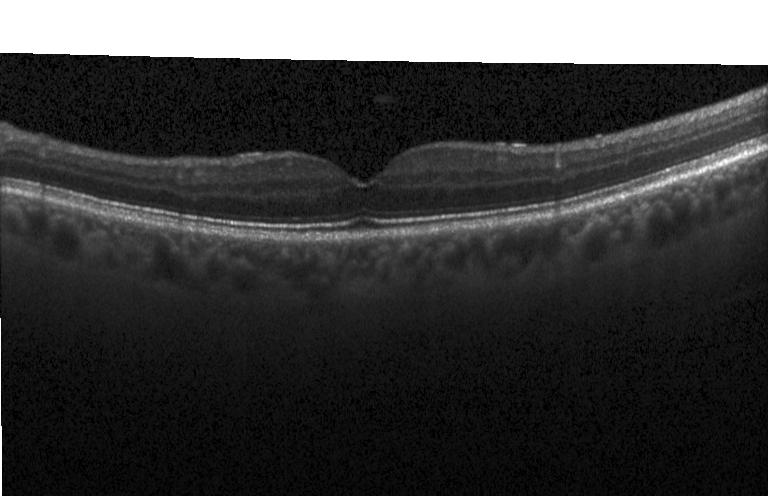

Spectral-domain OCT B-scan: no choroidal neovascularization, no diabetic macular edema, and no drusen.